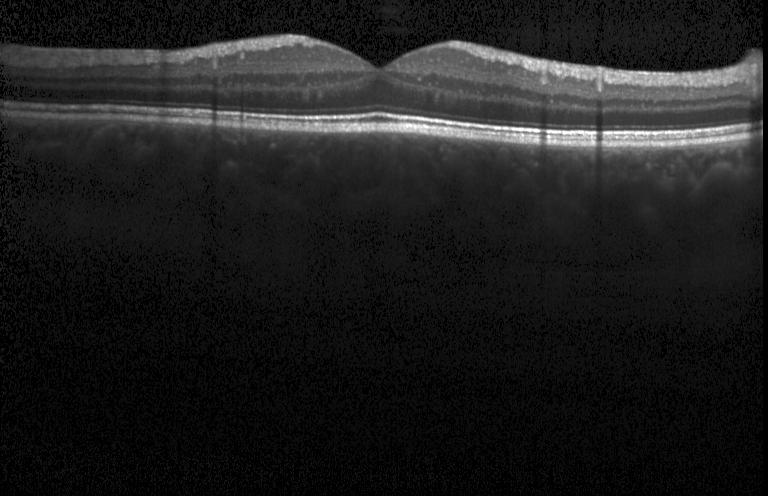 Centered on the fovea. Instrument: Heidelberg Spectralis. OCT B-scan. Diagnosis: neither choroidal neovascularization, diabetic macular edema, nor drusen.